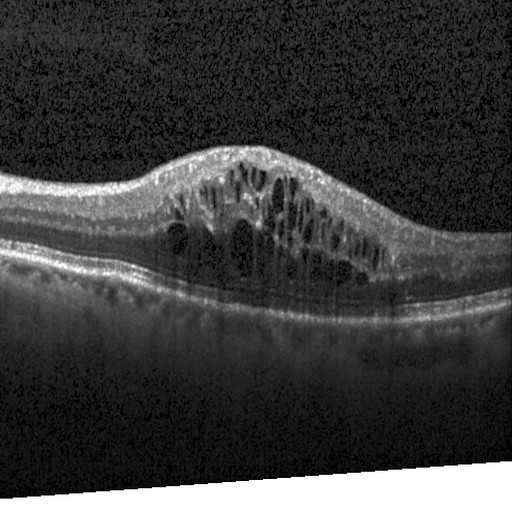
Finding: DME.